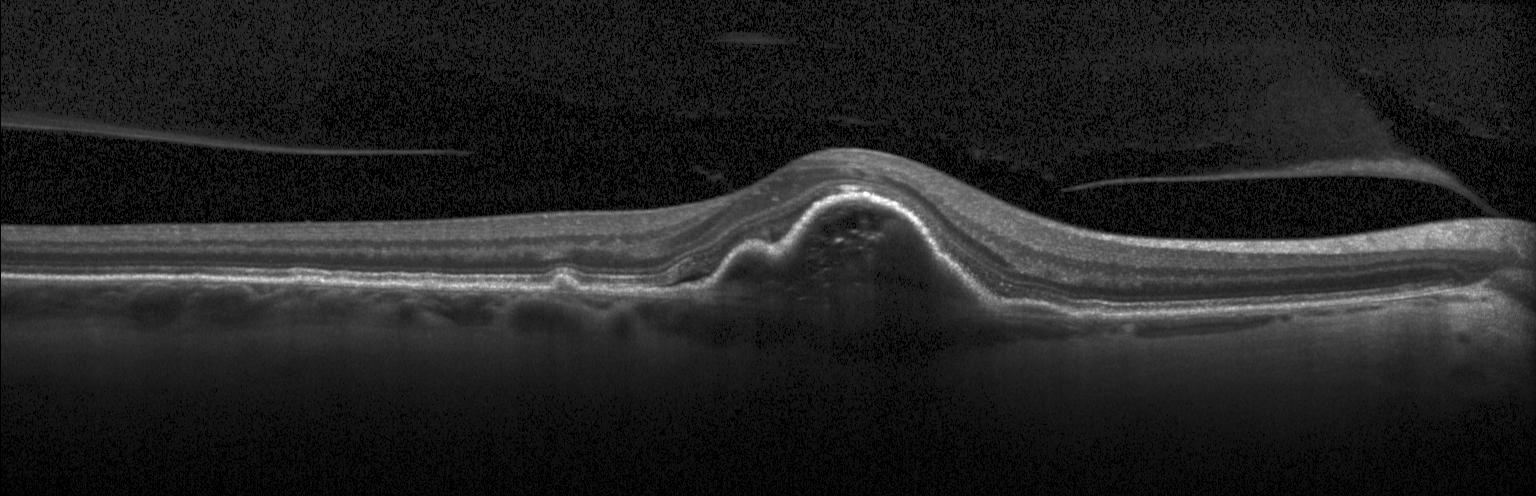

Assessment: choroidal neovascularization (CNV).